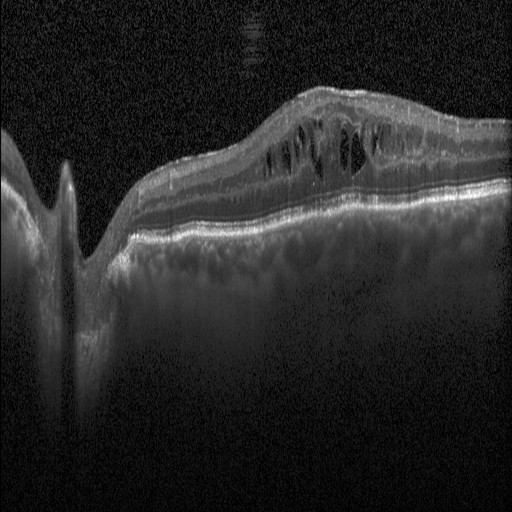

Centered on the fovea. Retinal OCT cross-section. Spectral-domain OCT.
Impression: diabetic macular edema.